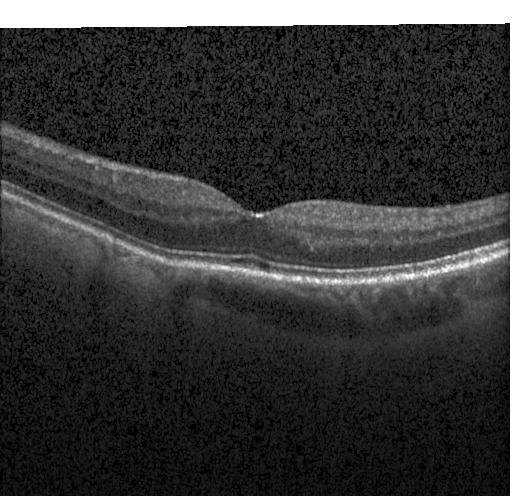

Retinal OCT cross-section
Finding: neither choroidal neovascularization, diabetic macular edema, nor drusen.